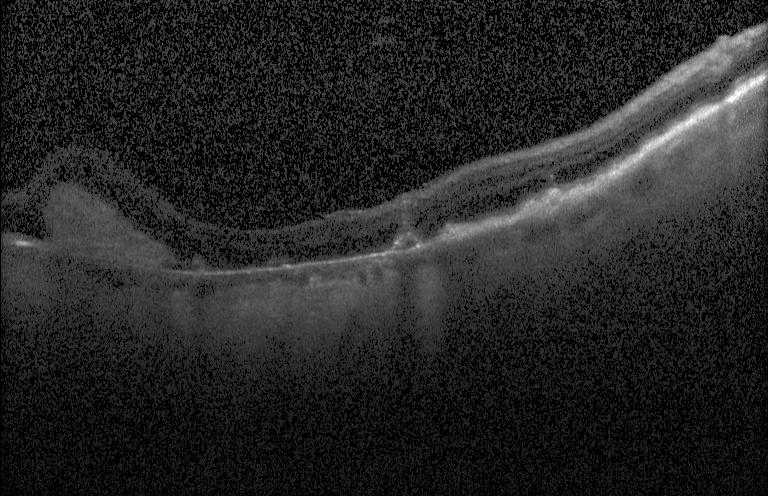 Finding: choroidal neovascularization (CNV).